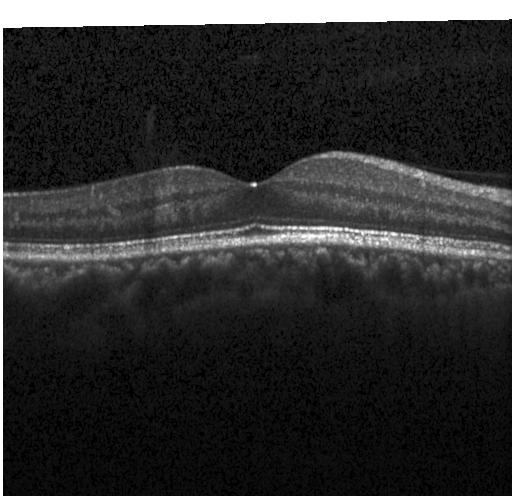

Retinal OCT cross-section, spectral-domain optical coherence tomography, macular scan. Impression: neither CNV, DME, nor drusen.